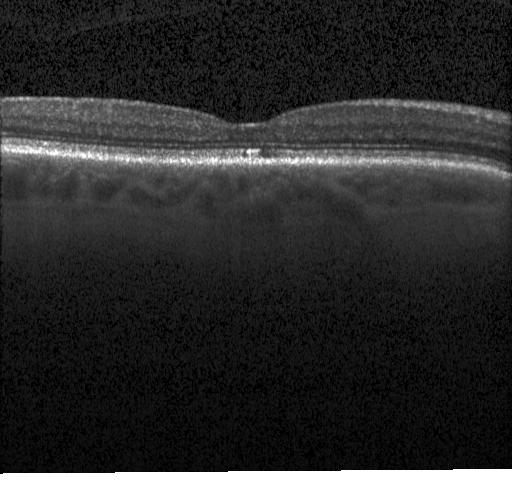

Optical coherence tomography scan — Neither CNV, DME, nor drusen.